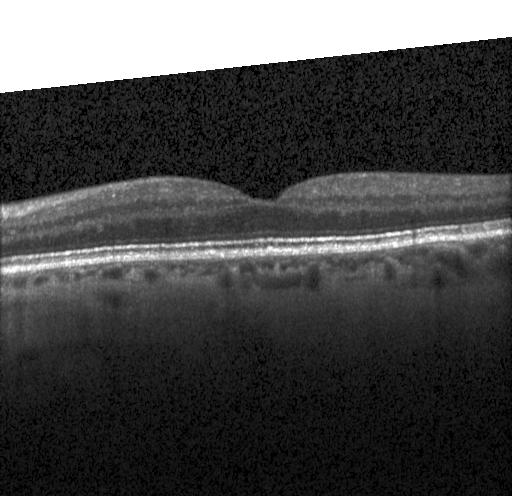

OCT finding: neither CNV, DME, nor drusen.